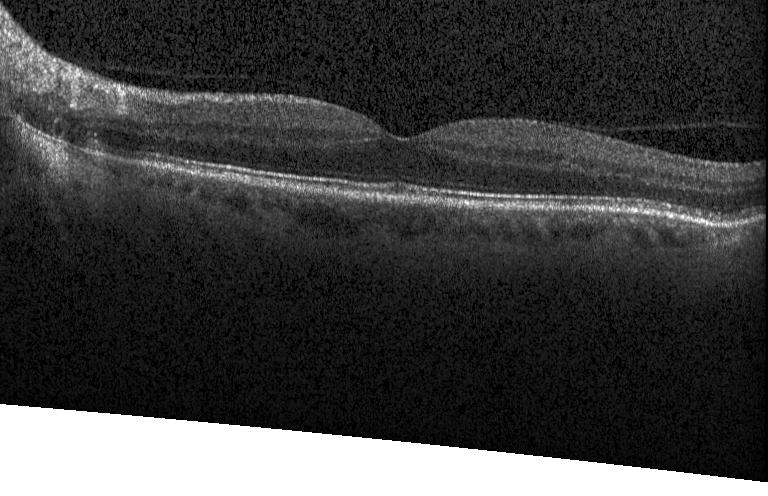
SD-OCT · retinal OCT B-scan
Dx: no evidence of CNV, DME, or drusen.